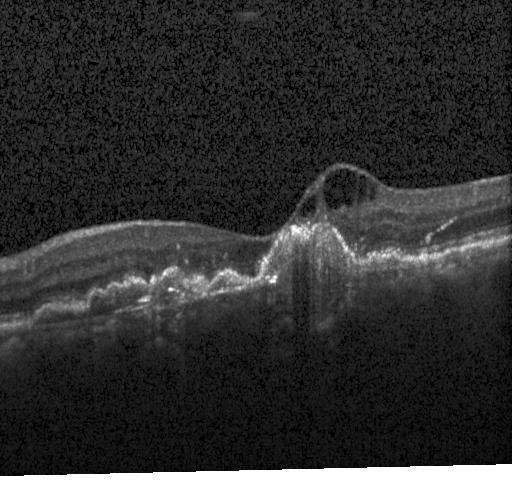
OCT B-scan showing a choroidal neovascular membrane.